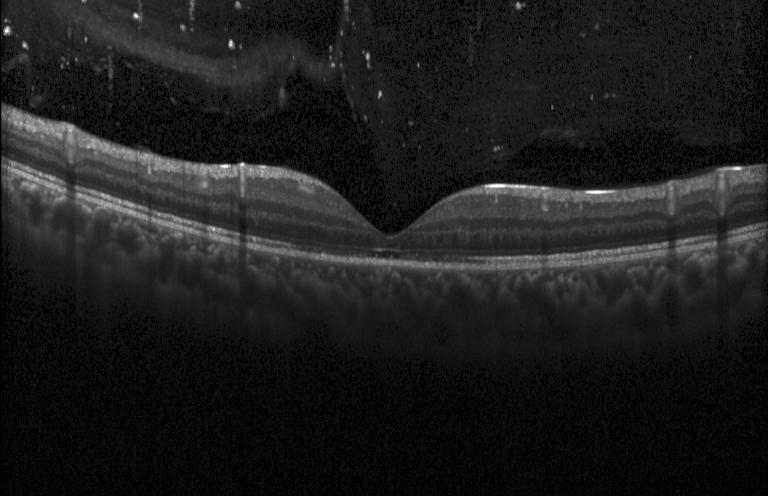 Through the macula, SD-OCT, optical coherence tomography B-scan — Assessment: neither choroidal neovascularization, diabetic macular edema, nor drusen.